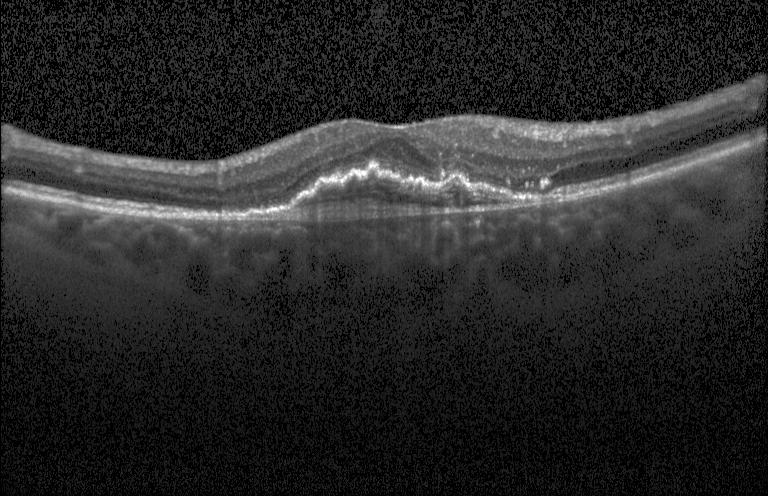 OCT finding: choroidal neovascularization.